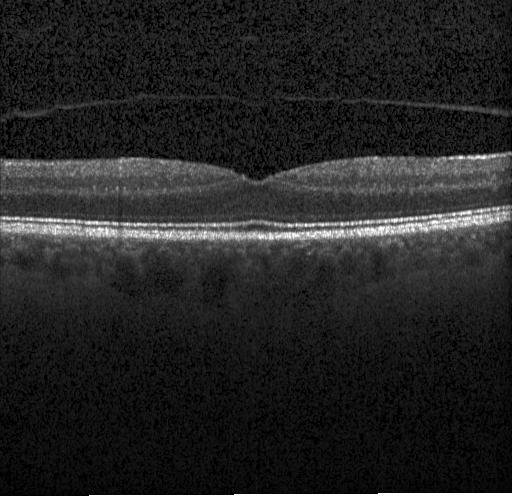
Diagnosis: no CNV, no DME, and no drusen.